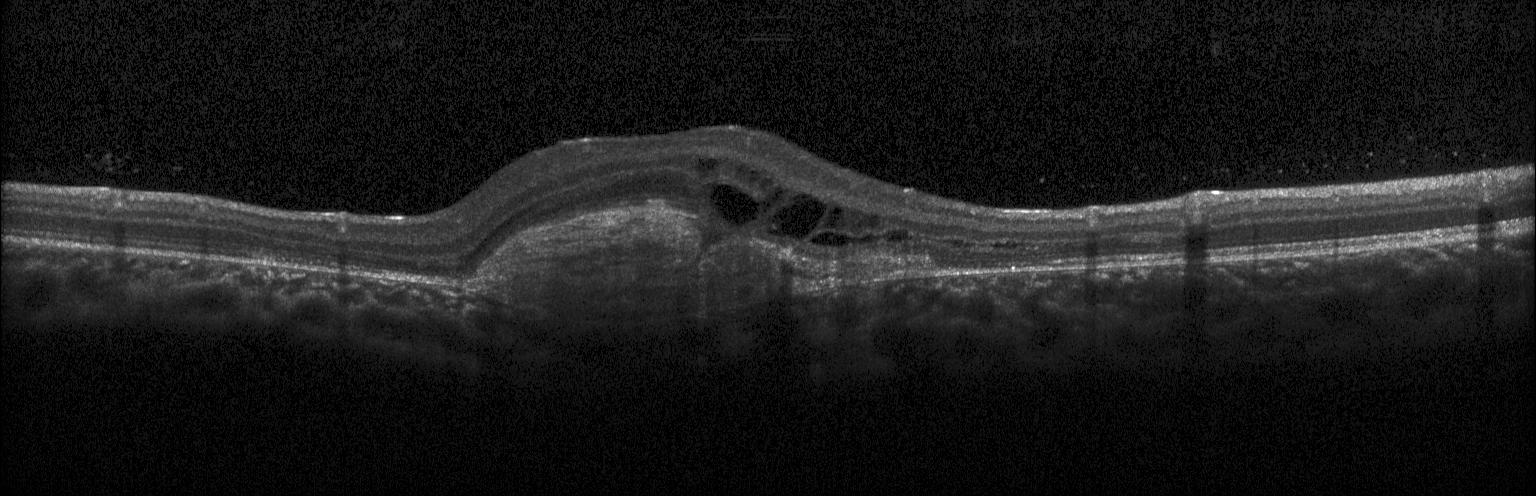
OCT B-scan, acquired on a Heidelberg Spectralis, fovea-centered.
OCT finding: choroidal neovascularization.